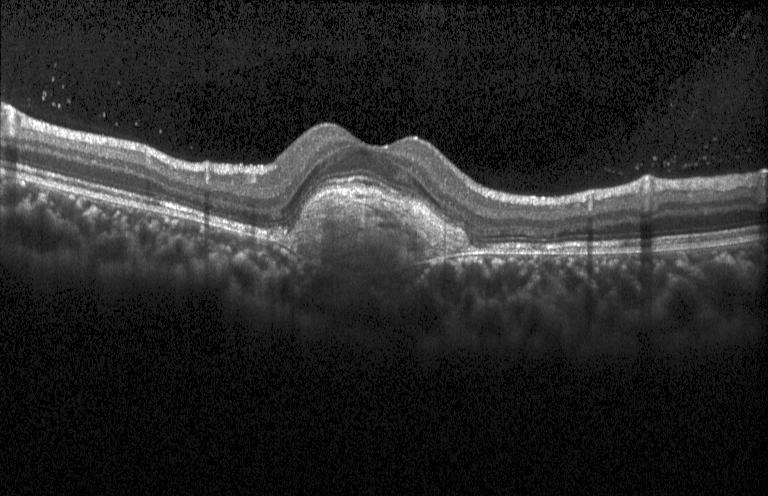

Optical coherence tomography B-scan. Impression: a choroidal neovascular membrane.